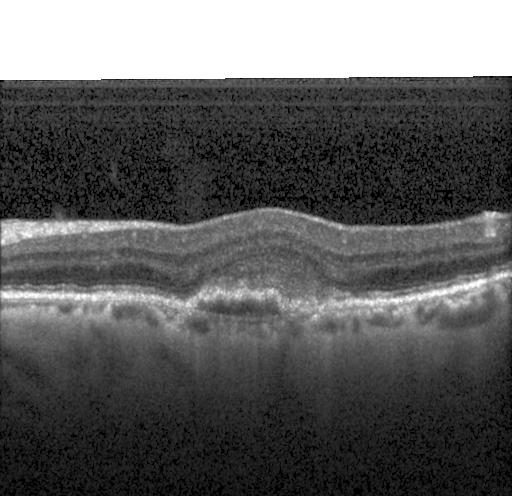

Optical coherence tomography scan · fovea-centered — Macular OCT: choroidal neovascularization (CNV).